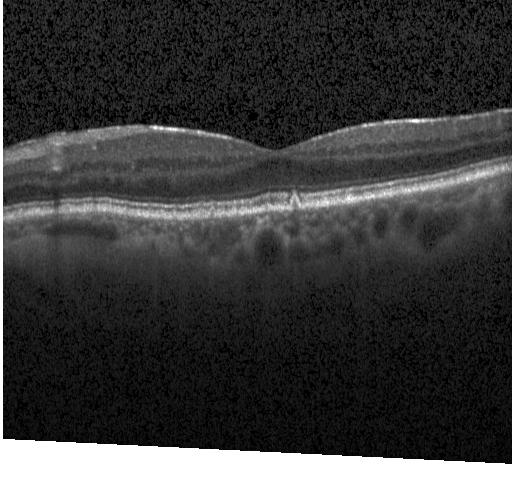 Spectral-domain OCT. OCT line scan. Heidelberg Spectralis OCT system.
Multiple drusen.